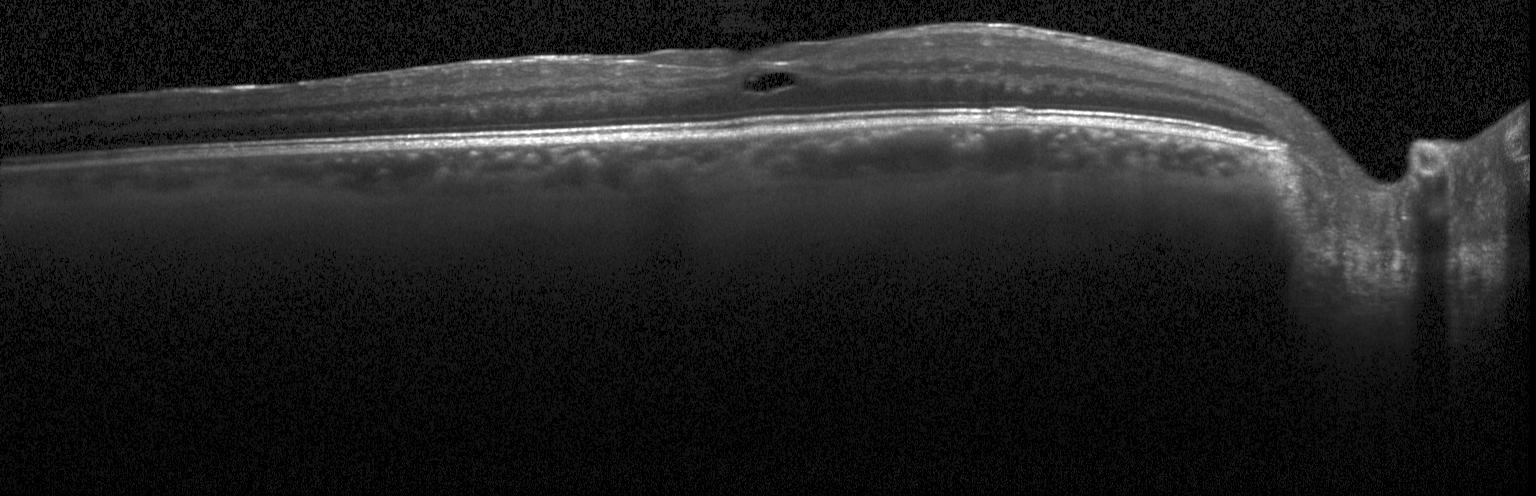

OCT finding: DME.